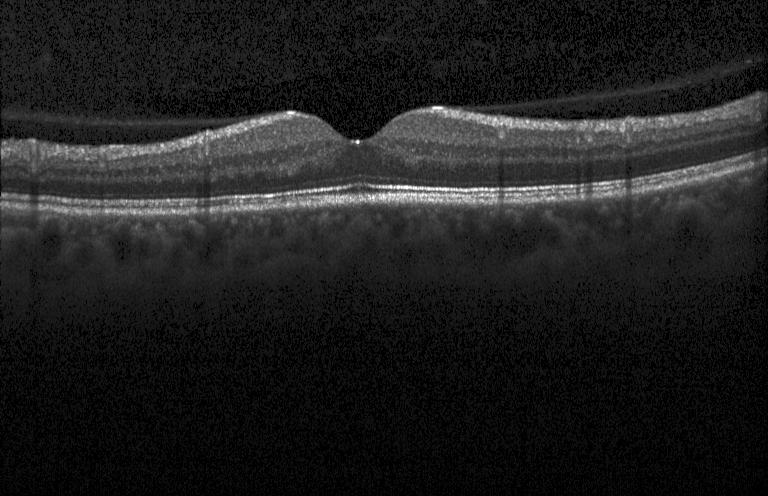

OCT B-scan showing no evidence of CNV, DME, or drusen.